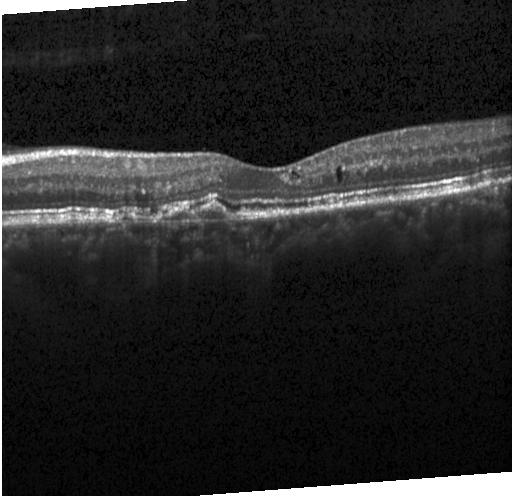 OCT finding: a choroidal neovascular membrane.